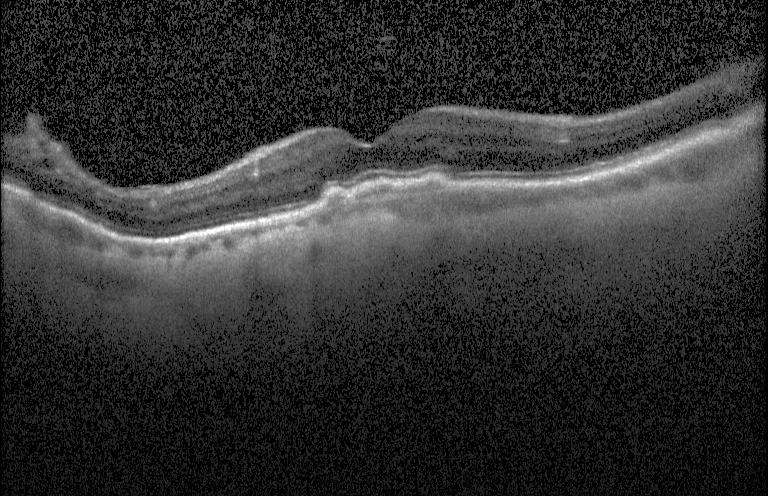

Optical coherence tomography B-scan — Impression: a choroidal neovascular membrane.